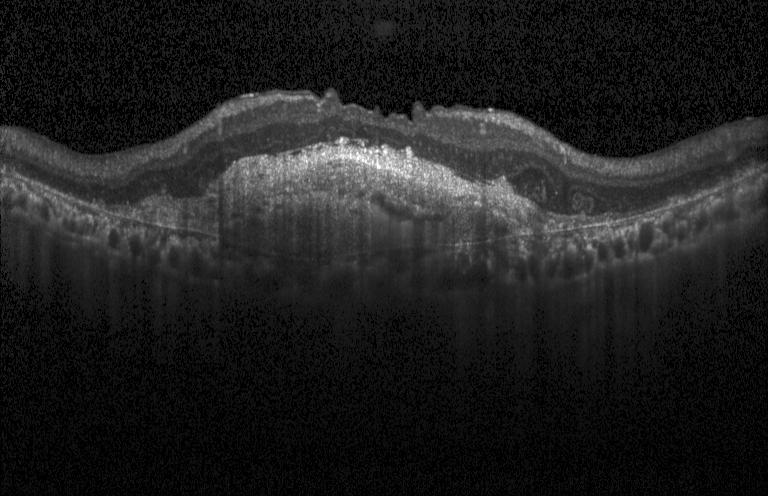
Diagnosis: a choroidal neovascular membrane.